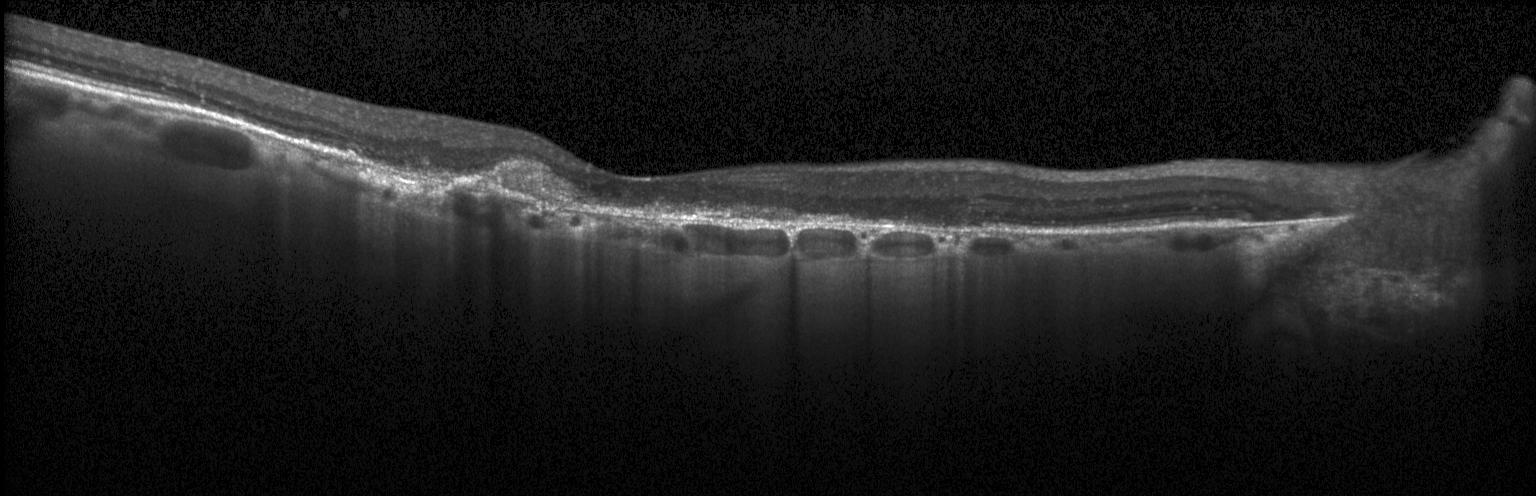

Retinal OCT B-scan — Diagnosis: a choroidal neovascular membrane.